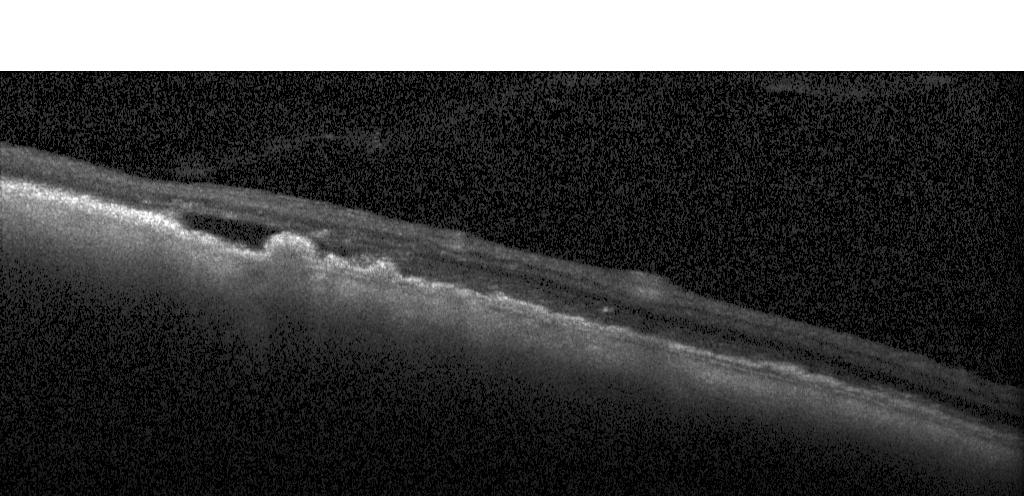
Retinal OCT B-scan
Assessment: a choroidal neovascular membrane.